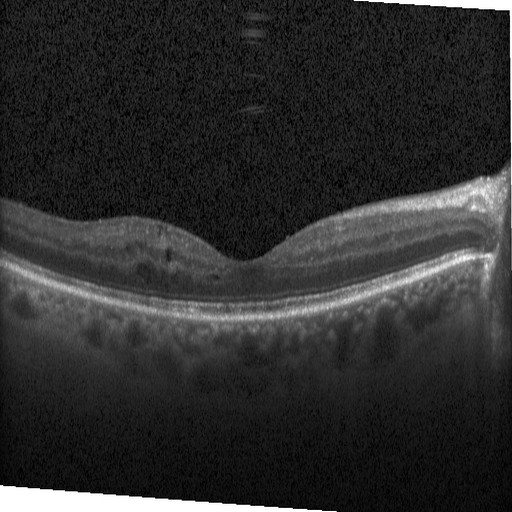
OCT line scan, fovea-centered.
Impression: diabetic macular edema.